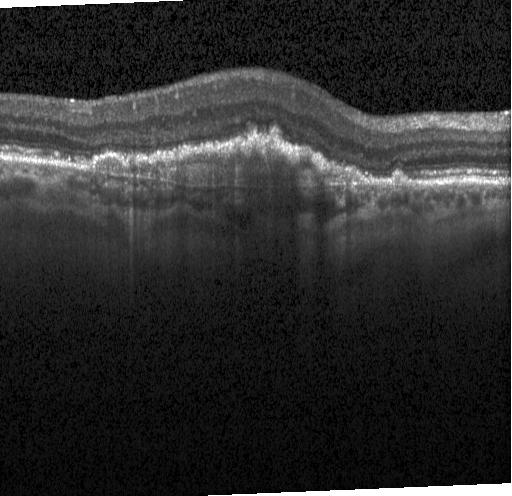 Instrument: Heidelberg Spectralis, horizontal scan through the fovea, optical coherence tomography B-scan
Diagnosis: a choroidal neovascular membrane.